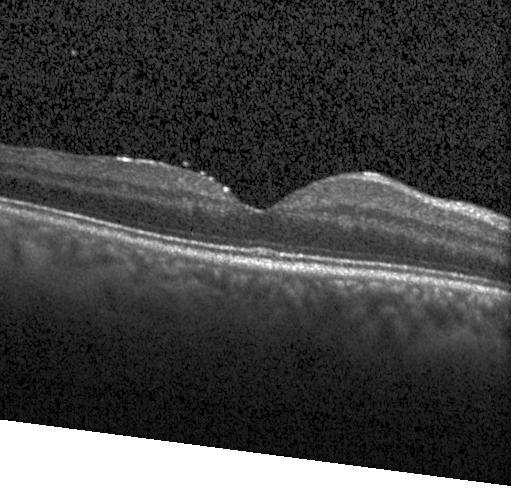

Fovea-centered · optical coherence tomography B-scan · Heidelberg Spectralis
Macular OCT: no choroidal neovascularization, diabetic macular edema, or drusen.